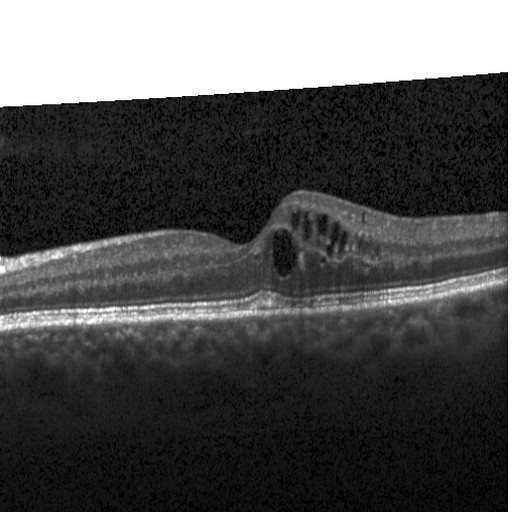

OCT B-scan; Heidelberg Spectralis OCT system — Impression: diabetic macular edema.